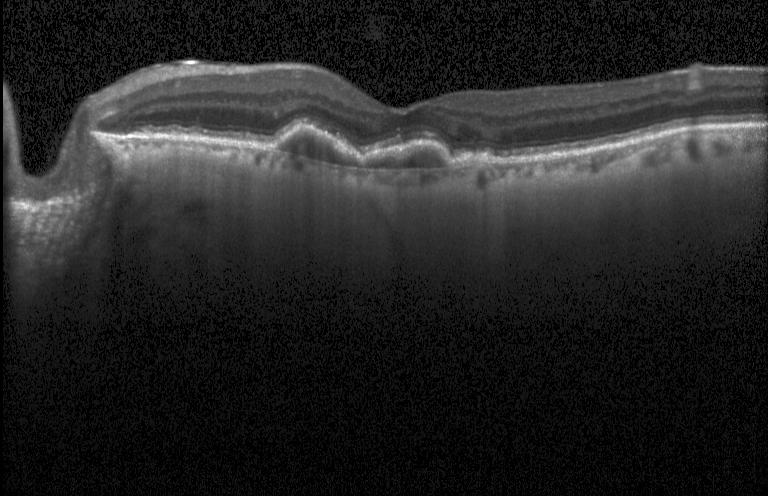

Diagnosis: choroidal neovascularization.